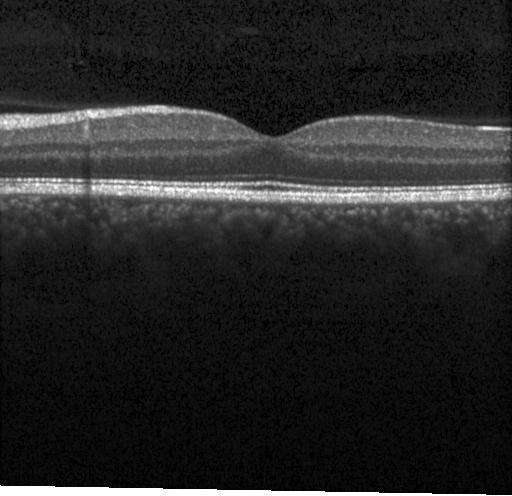
Assessment: no choroidal neovascularization, no diabetic macular edema, and no drusen.